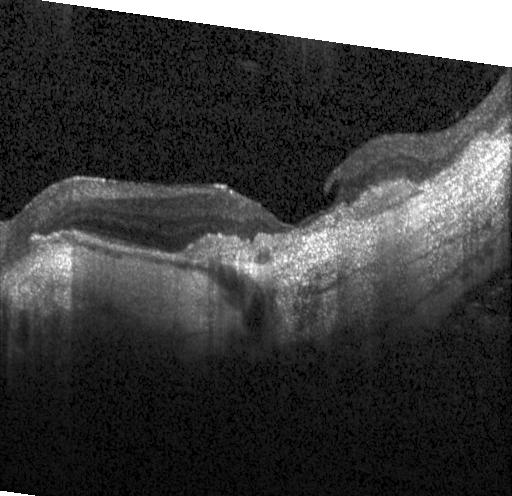

Retinal OCT cross-section. Impression: a choroidal neovascular membrane.